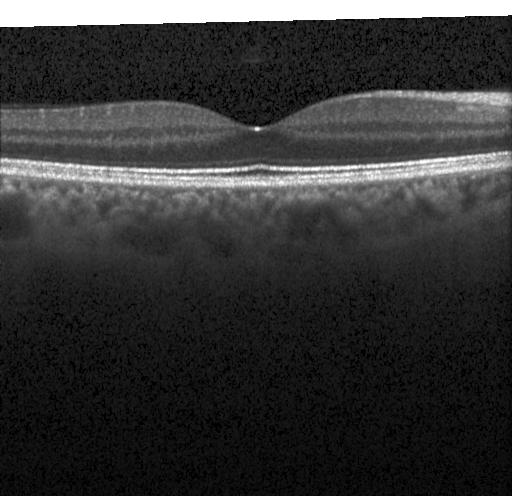
OCT line scan. Heidelberg Spectralis. Macular scan.
Diagnosis: no choroidal neovascularization, diabetic macular edema, or drusen.